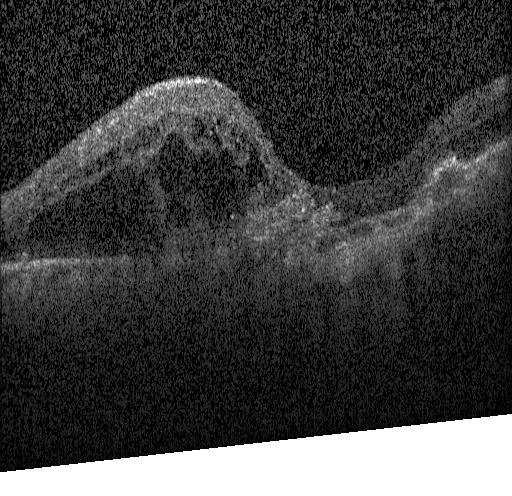 Assessment: a choroidal neovascular membrane.